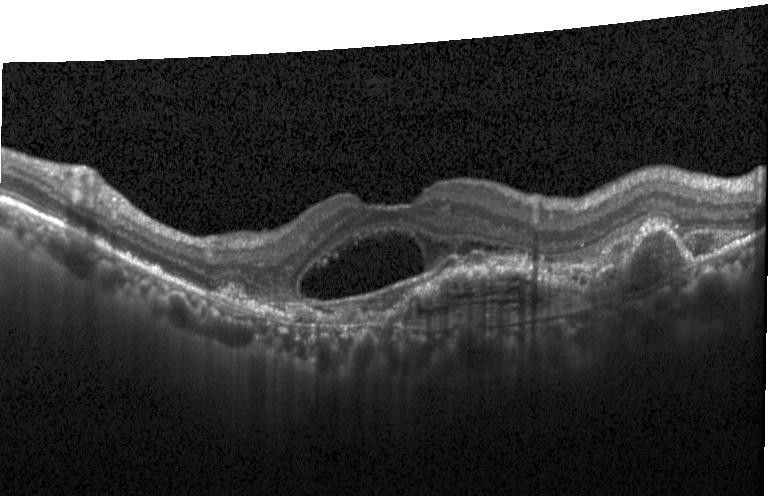 The scan shows a choroidal neovascular membrane.